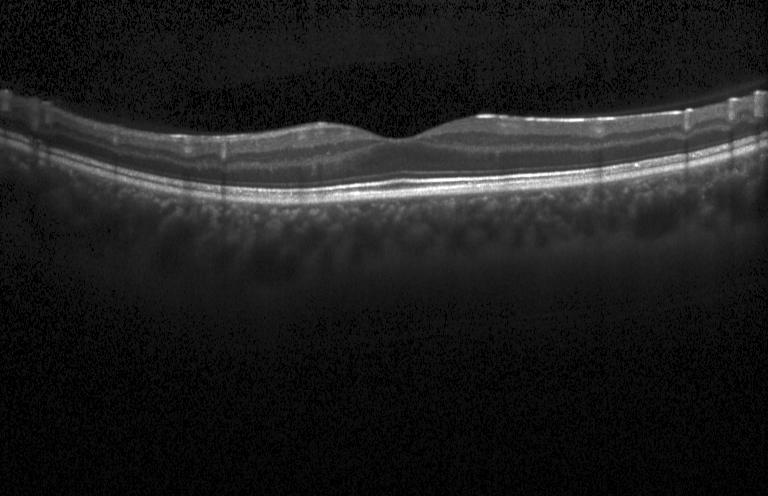

Retinal OCT cross-section
Assessment: no evidence of choroidal neovascularization, diabetic macular edema, or drusen.